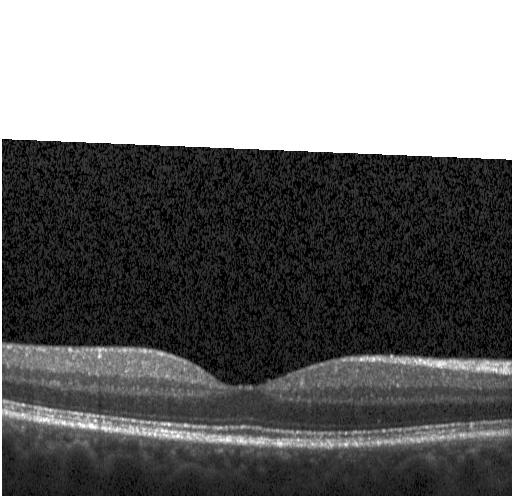

OCT scan showing no choroidal neovascularization, diabetic macular edema, or drusen.